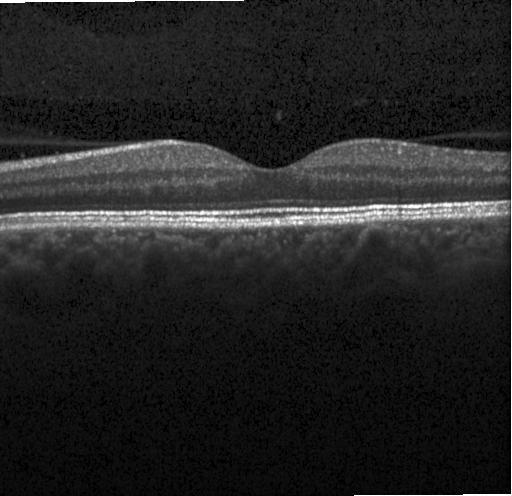

Impression: no evidence of choroidal neovascularization, diabetic macular edema, or drusen.